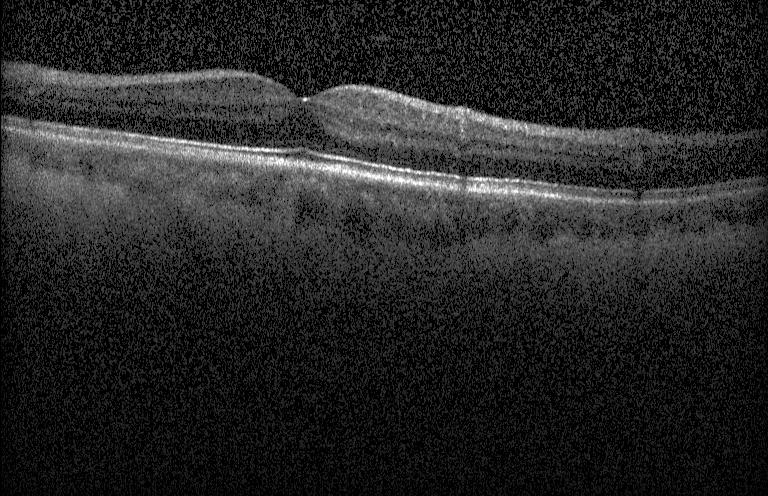

Dx: no choroidal neovascularization, no diabetic macular edema, and no drusen.